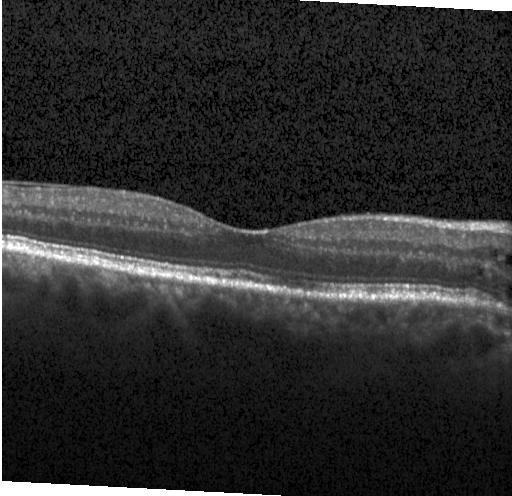 Optical coherence tomography B-scan.
Dx: DME.